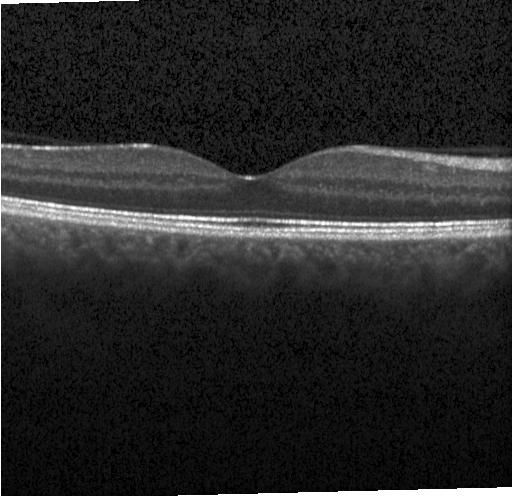

OCT line scan; spectral-domain OCT; fovea-centered. No evidence of choroidal neovascularization, diabetic macular edema, or drusen.